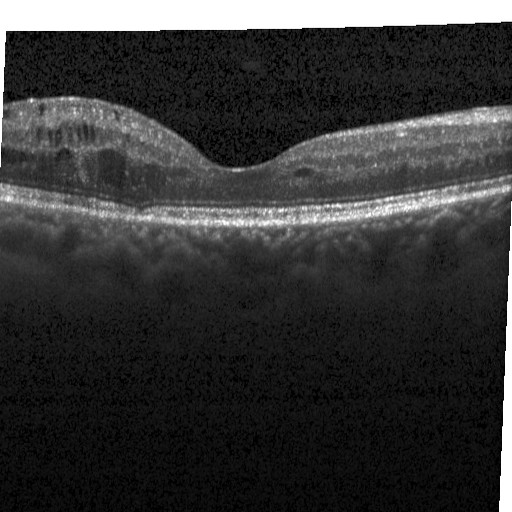 OCT B-scan. Dx: diabetic macular edema (DME).